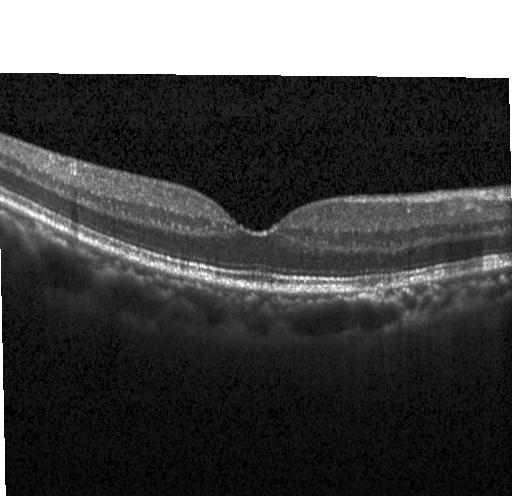
Optical coherence tomography B-scan
The scan shows no choroidal neovascularization, diabetic macular edema, or drusen.